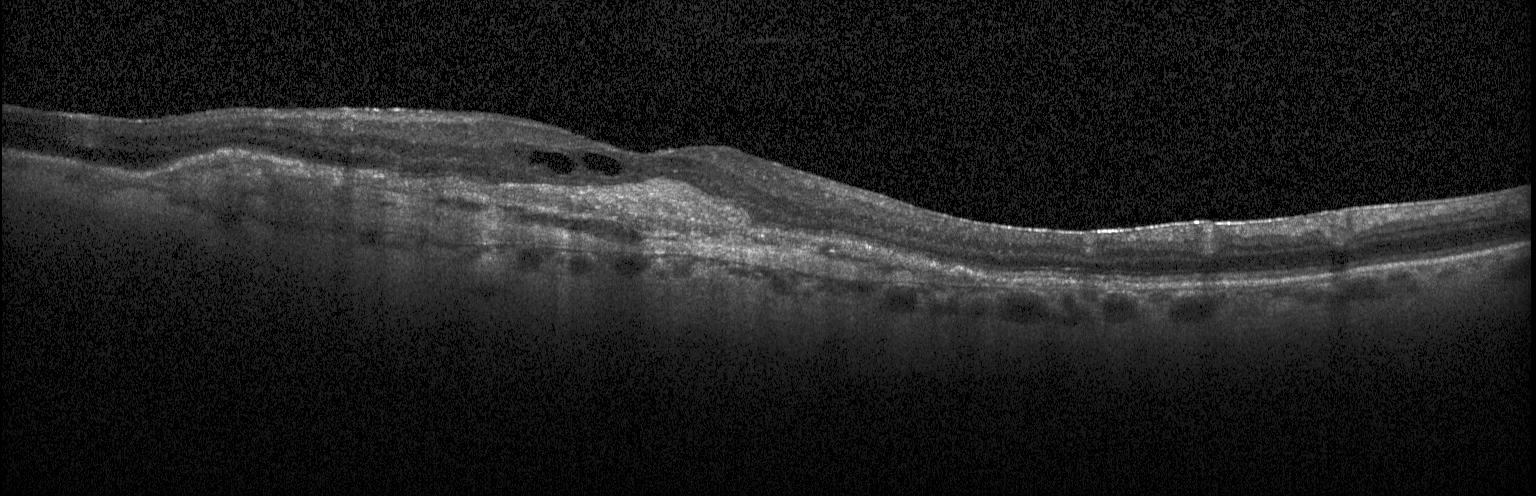 Heidelberg Spectralis OCT system, horizontal scan through the fovea, OCT line scan, spectral-domain OCT.
OCT finding: choroidal neovascularization (CNV).